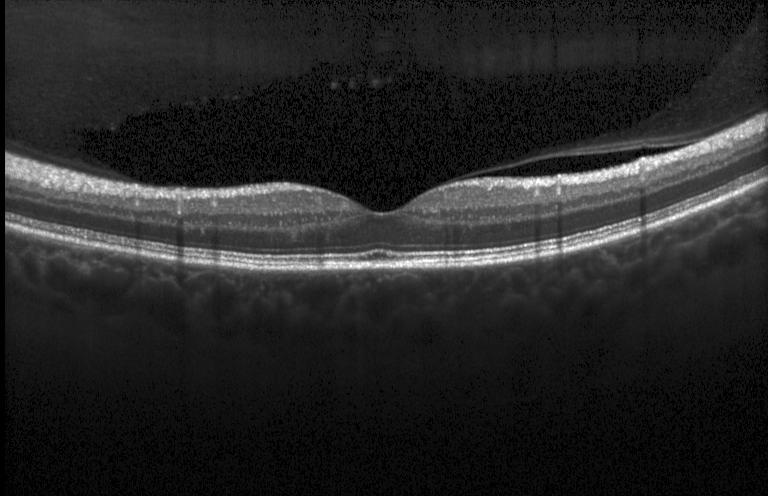
Retinal OCT cross-section. Fovea-centered
No evidence of choroidal neovascularization, diabetic macular edema, or drusen.